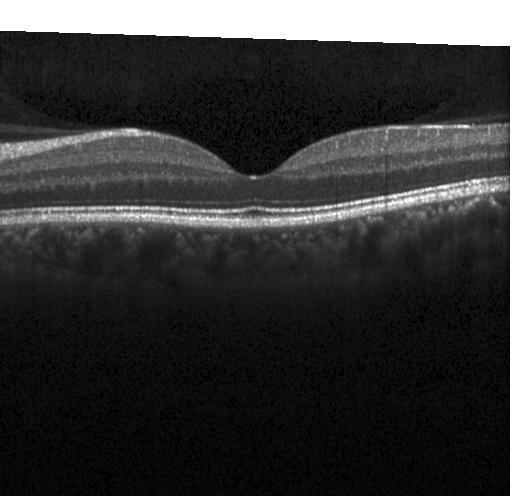 Fovea-centered. OCT line scan. Finding: no choroidal neovascularization, no diabetic macular edema, and no drusen.